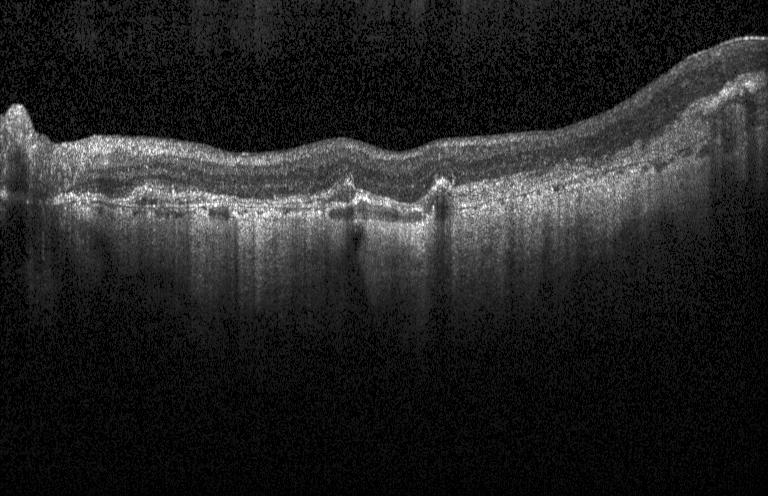
SD-OCT. Acquired on a Heidelberg Spectralis. Centered on the fovea. OCT line scan — The scan shows a choroidal neovascular membrane.